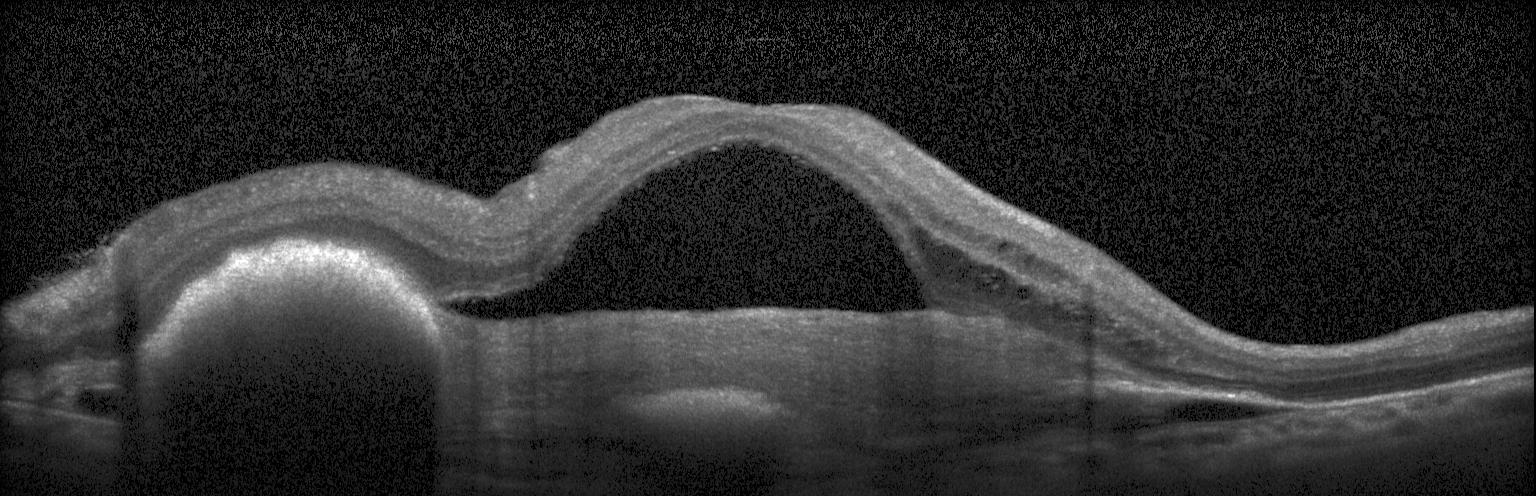 OCT line scan. Fovea-centered. SD-OCT — Finding: CNV.